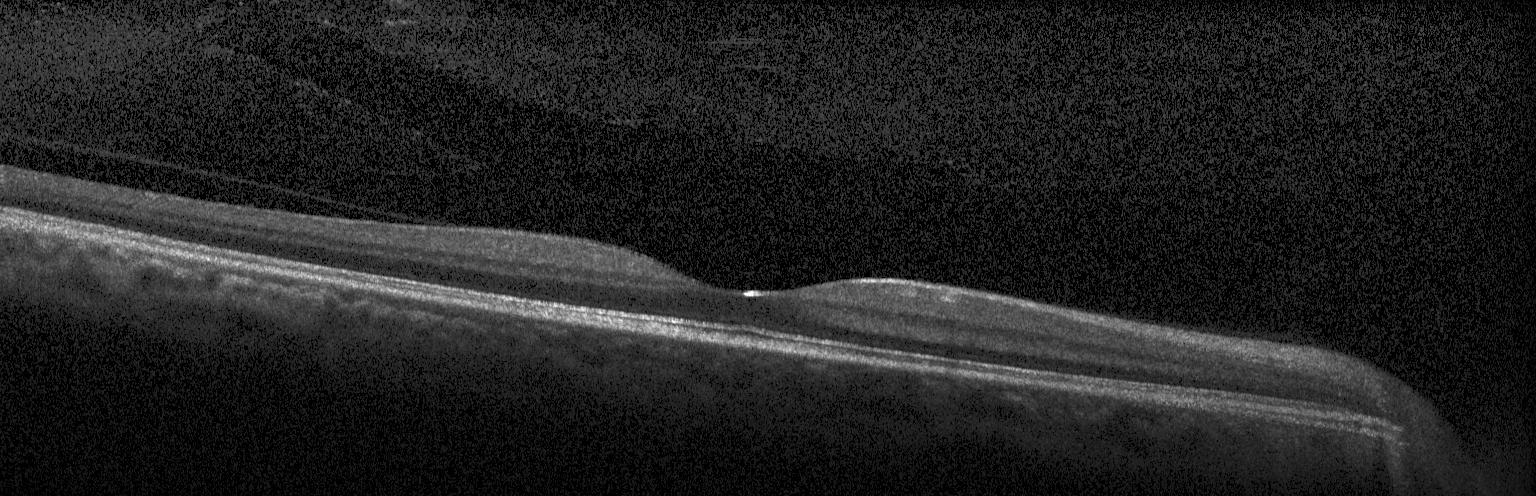

Assessment: no choroidal neovascularization, no diabetic macular edema, and no drusen.